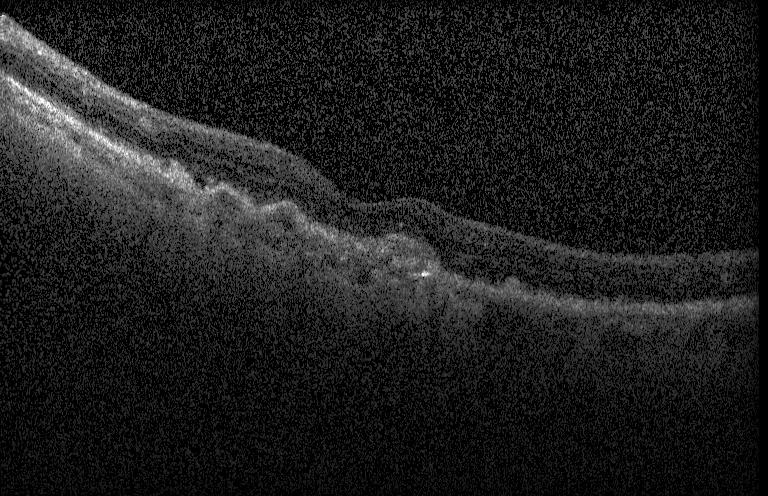
Optical coherence tomography B-scan · through the macula · spectral-domain optical coherence tomography · Heidelberg Spectralis OCT system
The scan shows CNV.